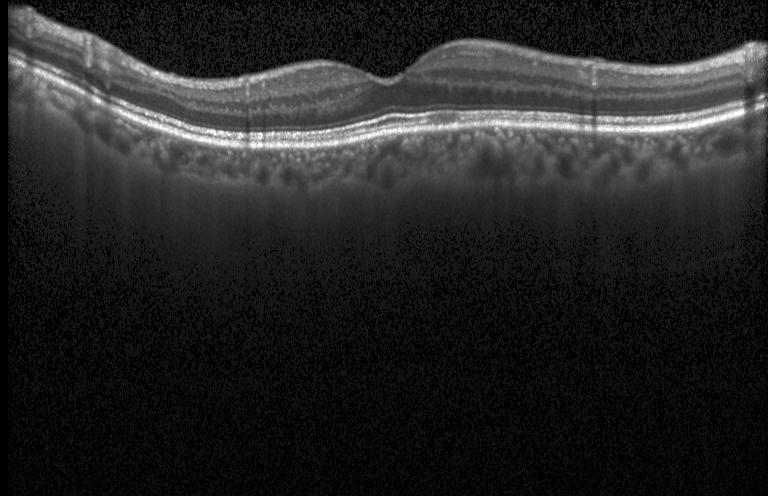

Macular OCT: no choroidal neovascularization, no diabetic macular edema, and no drusen.